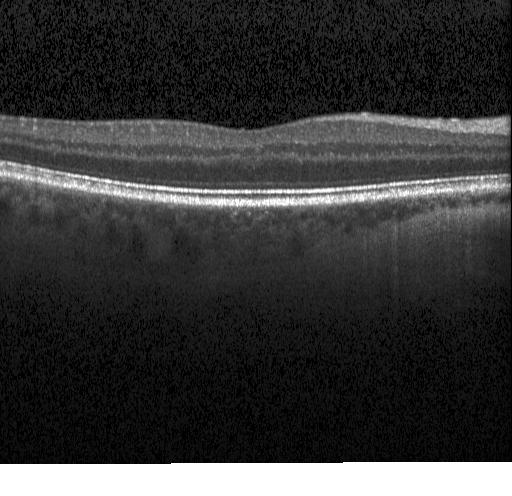 Horizontal scan through the fovea, OCT line scan — Dx: neither choroidal neovascularization, diabetic macular edema, nor drusen.